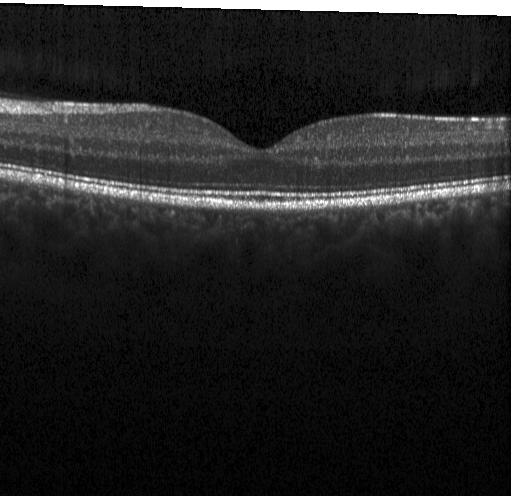 Acquired on a Heidelberg Spectralis, retinal OCT B-scan.
Diagnosis: neither CNV, DME, nor drusen.